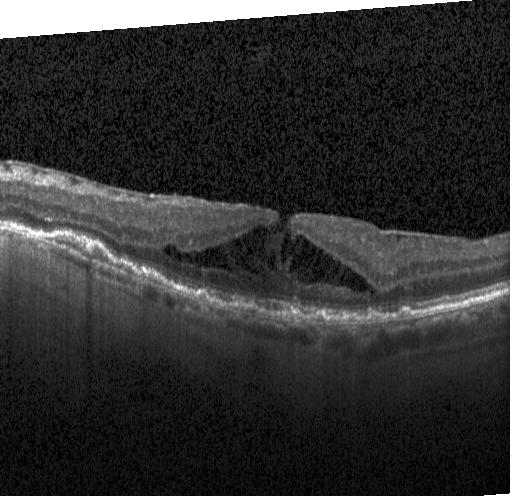

OCT line scan — Macular OCT: diabetic macular edema (DME).